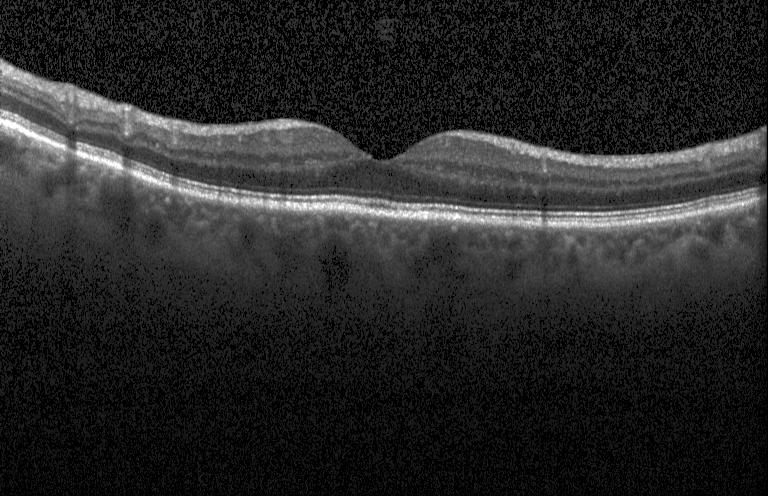 Spectral-domain OCT B-scan: no evidence of choroidal neovascularization, diabetic macular edema, or drusen.